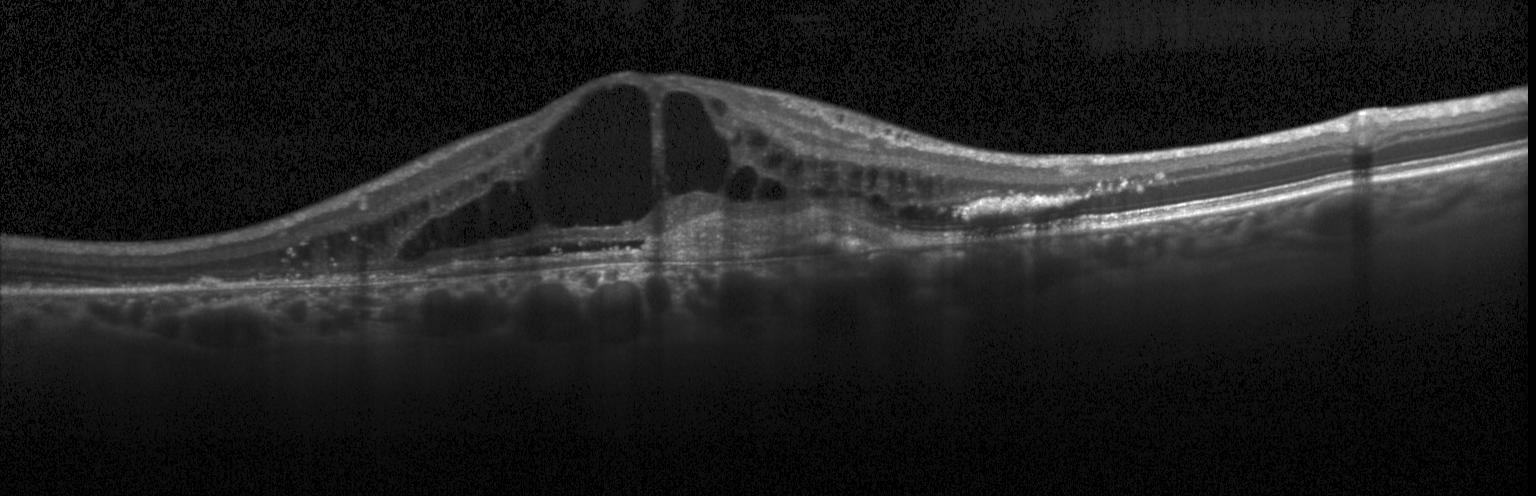

Impression: choroidal neovascularization (CNV).